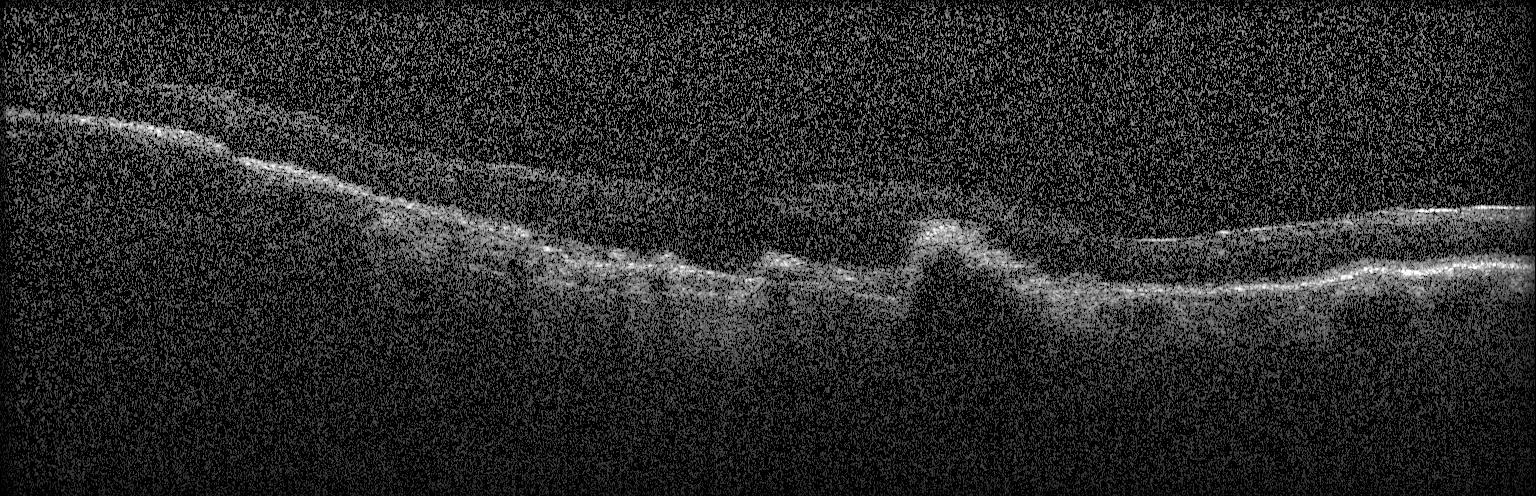

Heidelberg Spectralis OCT system, optical coherence tomography scan — Impression: CNV.